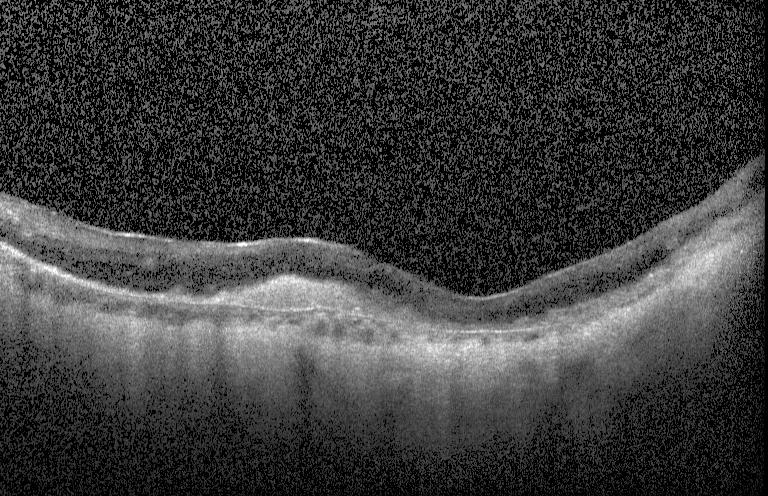 OCT line scan — Impression: choroidal neovascularization.